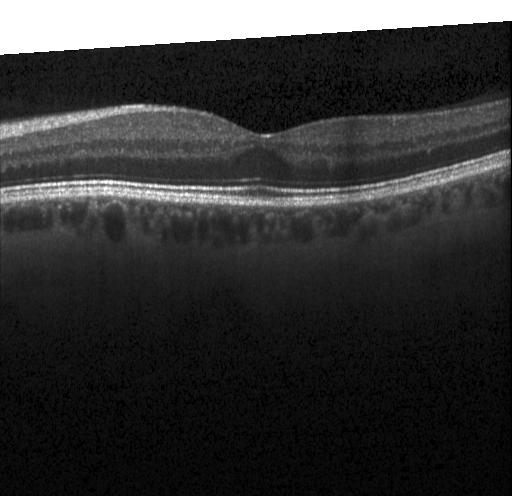
Instrument: Heidelberg Spectralis · OCT line scan · SD-OCT
Assessment: neither CNV, DME, nor drusen.